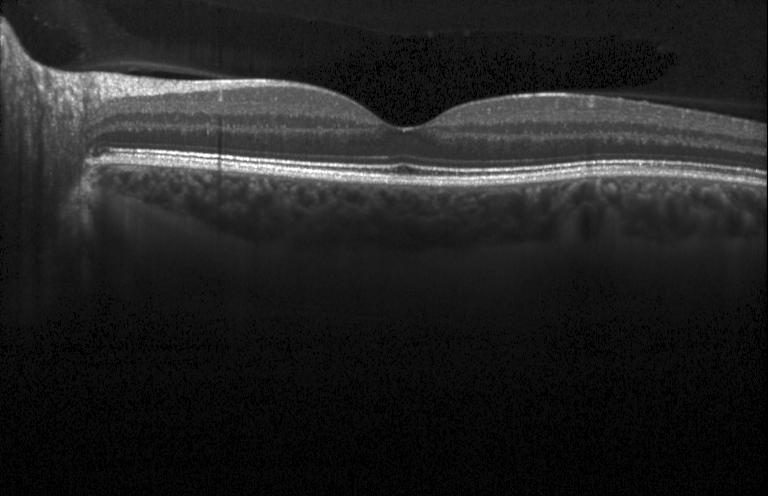 This B-scan demonstrates neither choroidal neovascularization, diabetic macular edema, nor drusen.